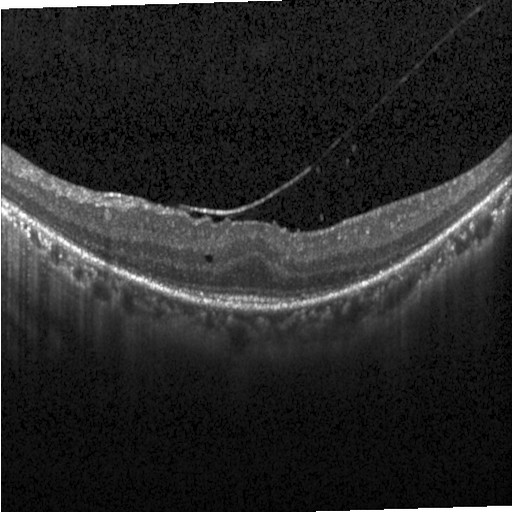
Macular OCT: diabetic macular edema (DME).